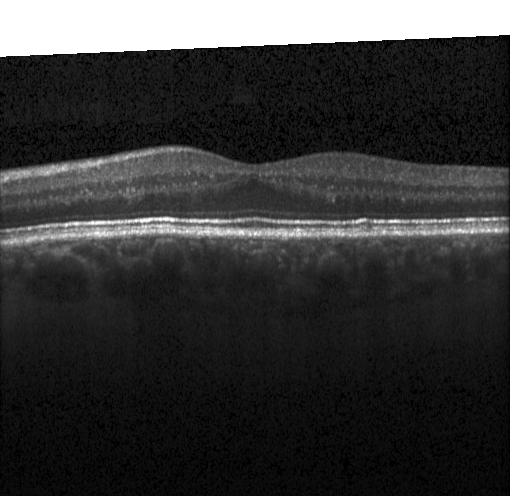 OCT B-scan
Assessment: no choroidal neovascularization, diabetic macular edema, or drusen.